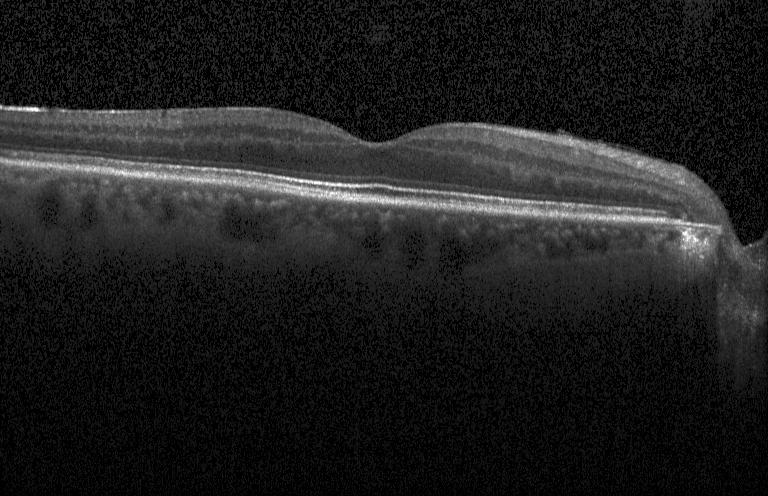
Finding: neither choroidal neovascularization, diabetic macular edema, nor drusen.